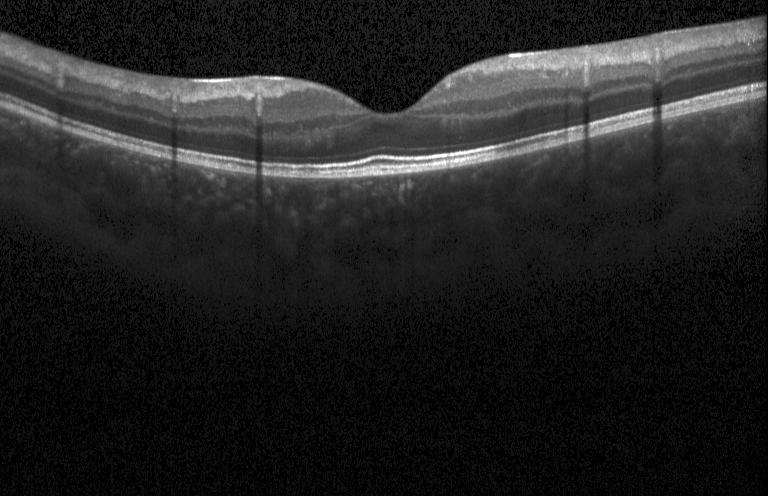 Retinal OCT cross-section showing no evidence of choroidal neovascularization, diabetic macular edema, or drusen.